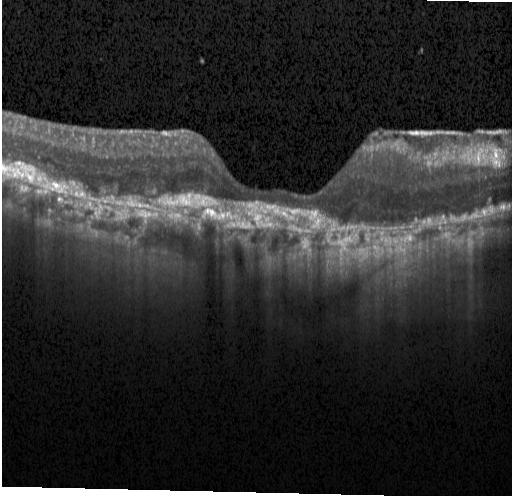

OCT line scan, Heidelberg Spectralis, centered on the fovea.
OCT finding: a choroidal neovascular membrane.